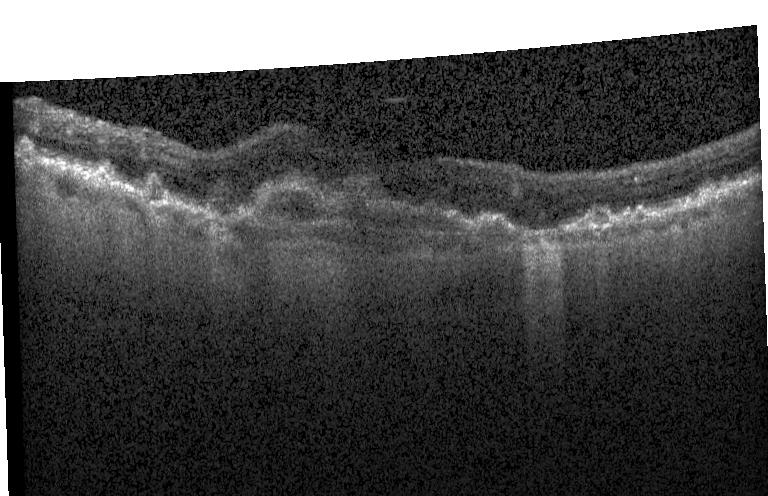

OCT line scan. Macular scan. Acquired on a Heidelberg Spectralis. SD-OCT — Finding: a choroidal neovascular membrane.